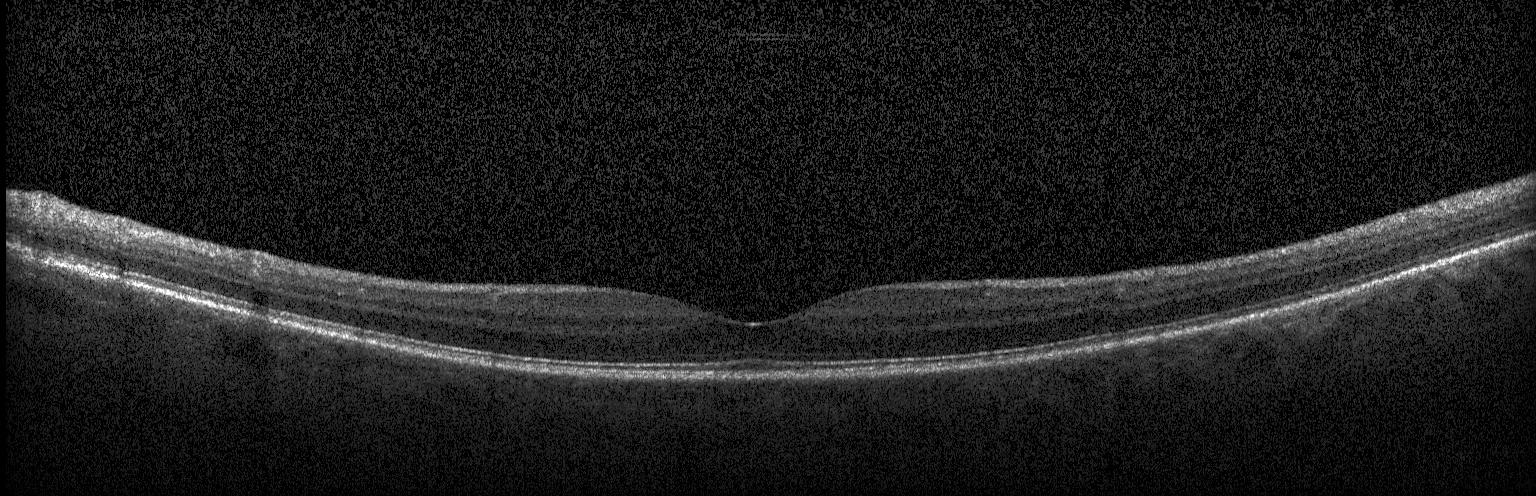

Through the macula. Heidelberg Spectralis OCT system. SD-OCT. Retinal OCT B-scan.
OCT finding: no CNV, DME, or drusen.